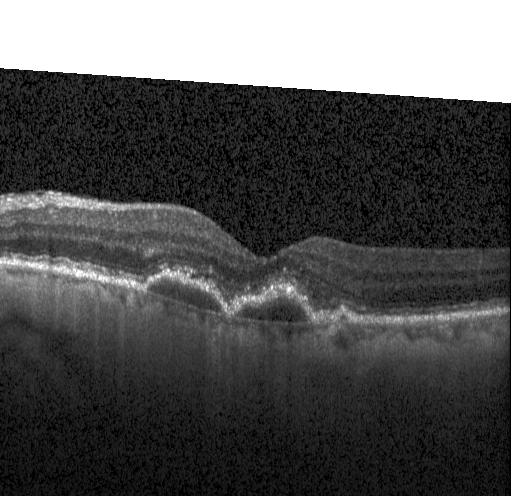

SD-OCT, macular scan, instrument: Heidelberg Spectralis, optical coherence tomography B-scan — Finding: a choroidal neovascular membrane.